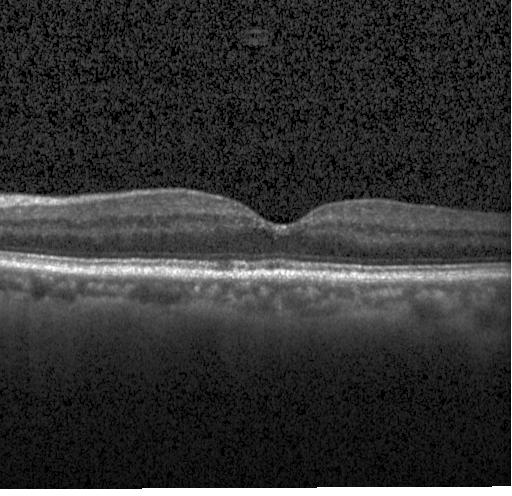
Spectral-domain OCT B-scan: neither choroidal neovascularization, diabetic macular edema, nor drusen.